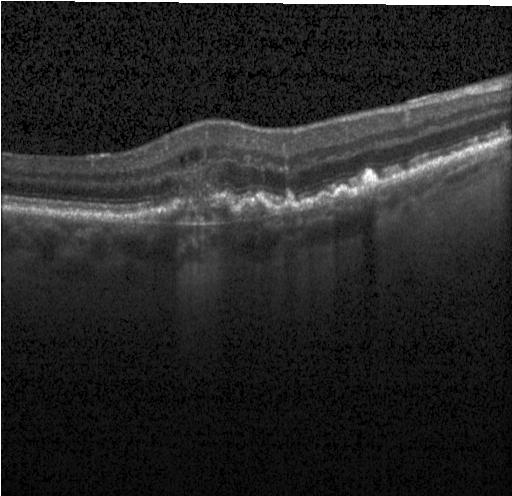

Horizontal scan through the fovea. Heidelberg Spectralis. Retinal OCT cross-section. Finding: a choroidal neovascular membrane.